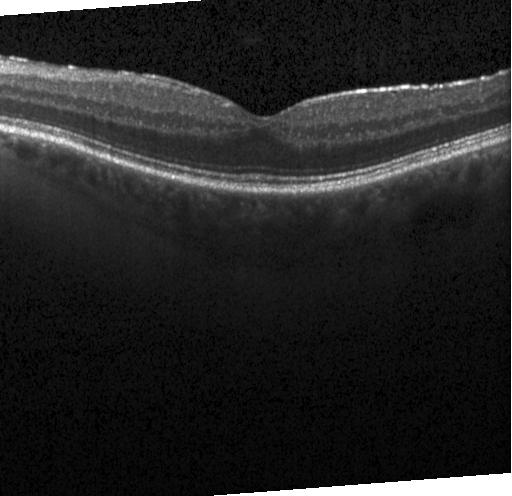 Retinal OCT B-scan. Heidelberg Spectralis OCT system. Finding: no choroidal neovascularization, no diabetic macular edema, and no drusen.